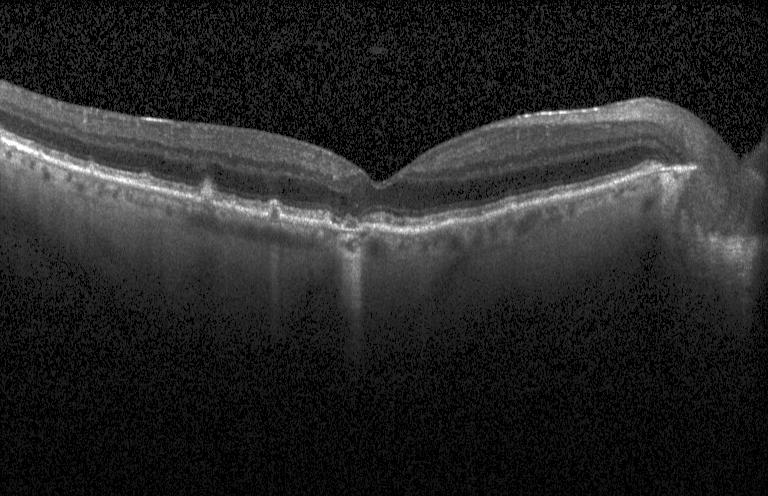 Finding: sub-RPE drusenoid deposits.